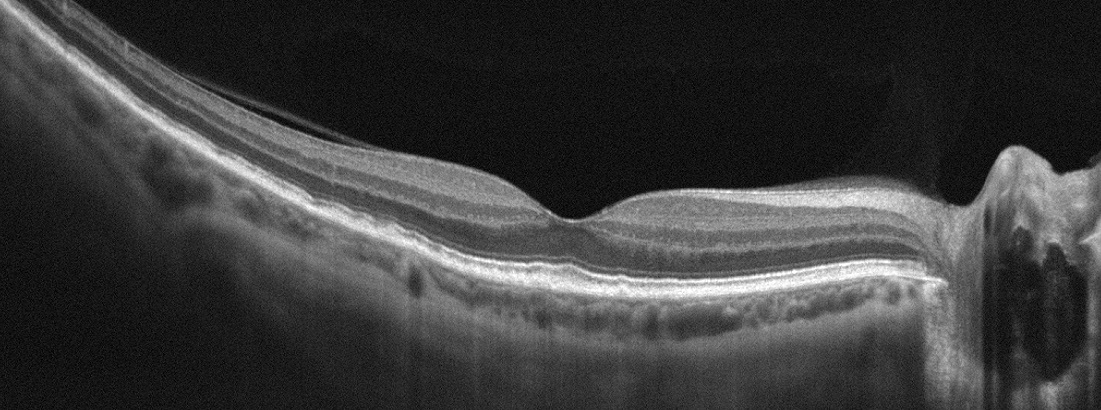
Dx: age-related macular degeneration.